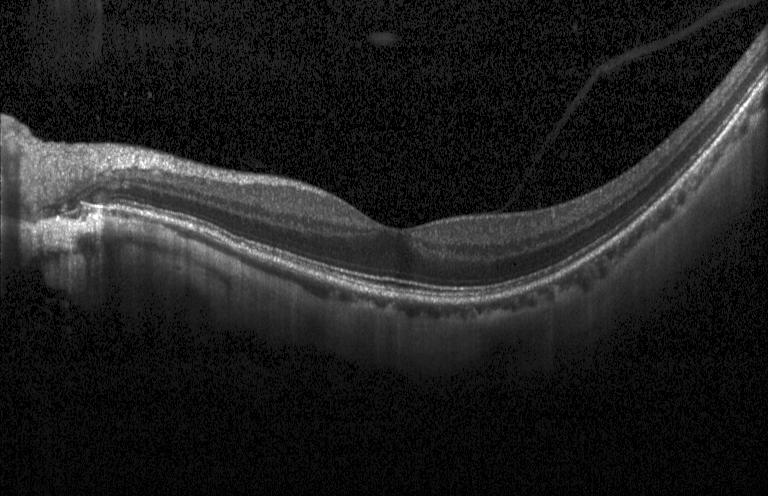 Diagnosis: no CNV, DME, or drusen.